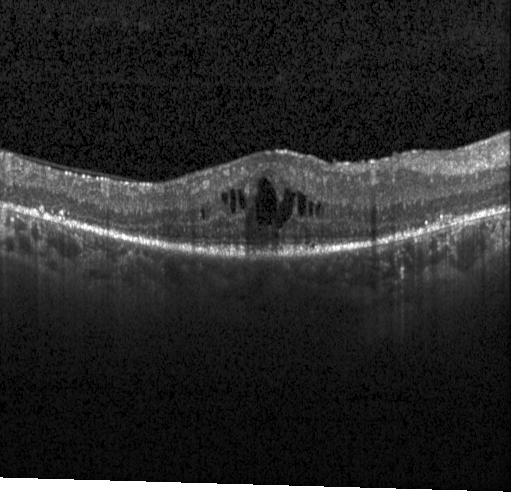 Spectral-domain optical coherence tomography. OCT B-scan. Through the macula — Macular OCT: DME.